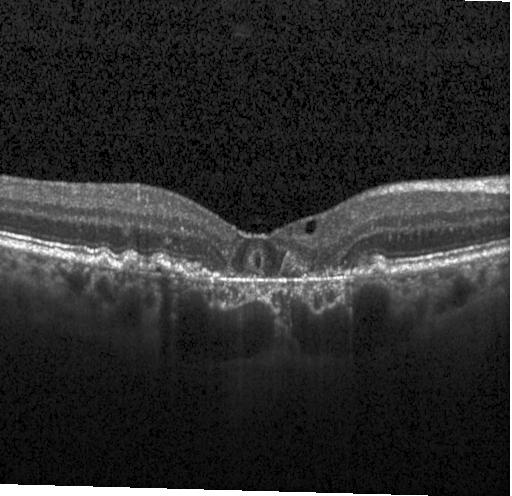

Macular OCT: a choroidal neovascular membrane.